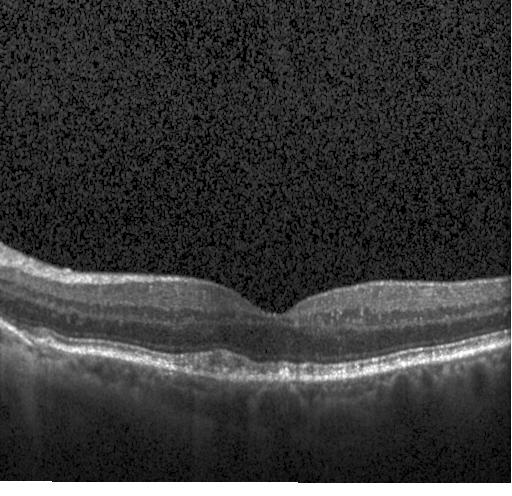

Finding: sub-RPE drusenoid deposits.